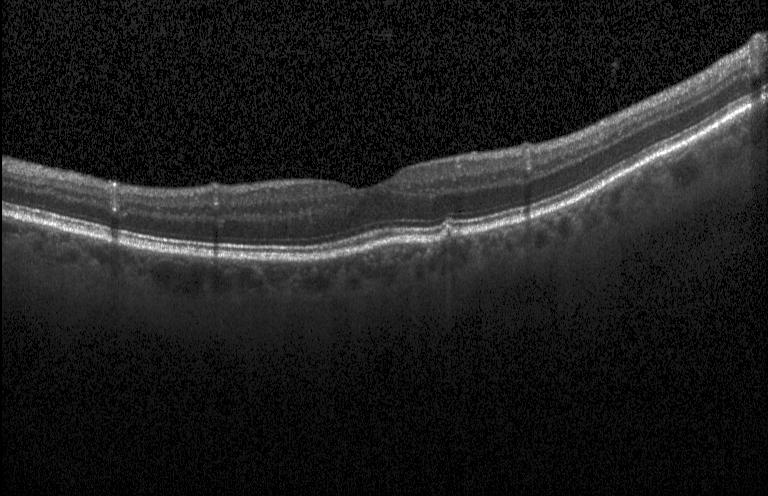

Heidelberg Spectralis OCT system, retinal OCT B-scan, spectral-domain optical coherence tomography, through the macula
Finding: sub-RPE drusenoid deposits.